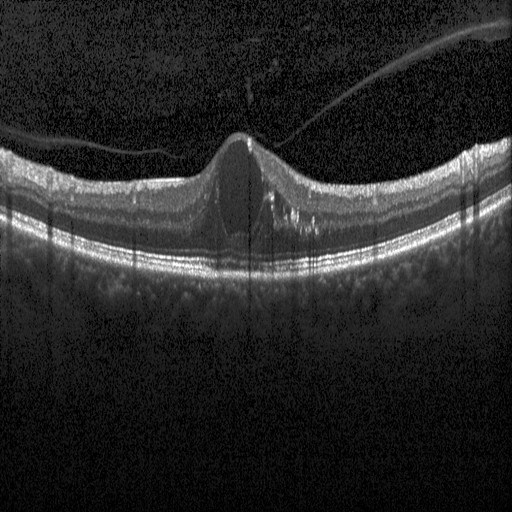
Macular OCT demonstrating DME.